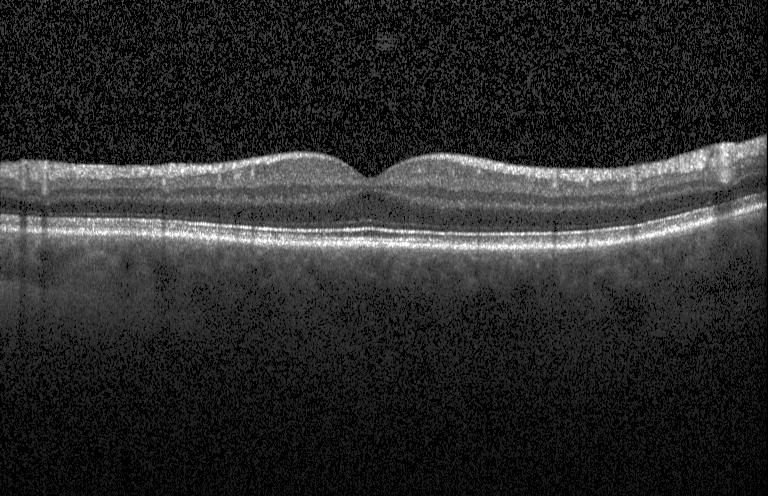
Spectral-domain optical coherence tomography. Acquired on a Heidelberg Spectralis. OCT line scan. Centered on the fovea
Finding: no evidence of choroidal neovascularization, diabetic macular edema, or drusen.